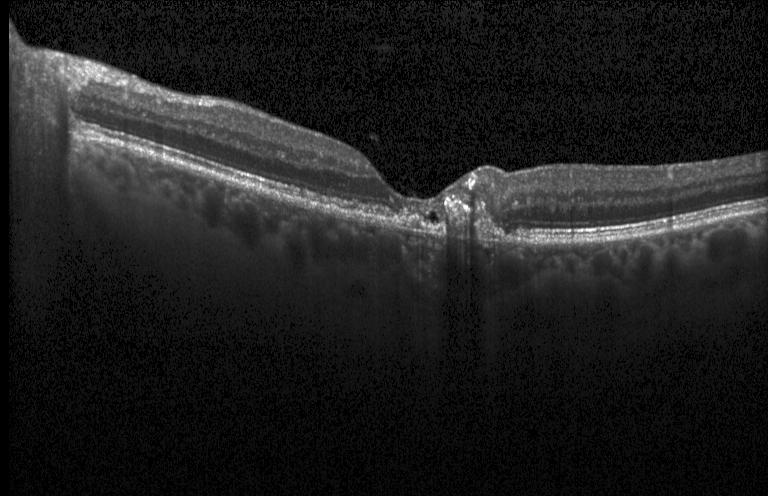
Impression: a choroidal neovascular membrane.